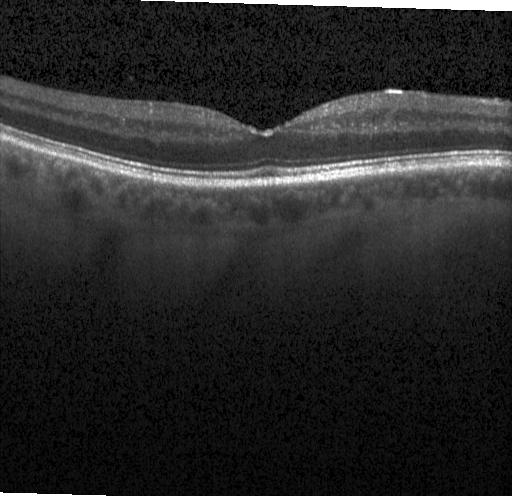
Macular OCT: neither CNV, DME, nor drusen.